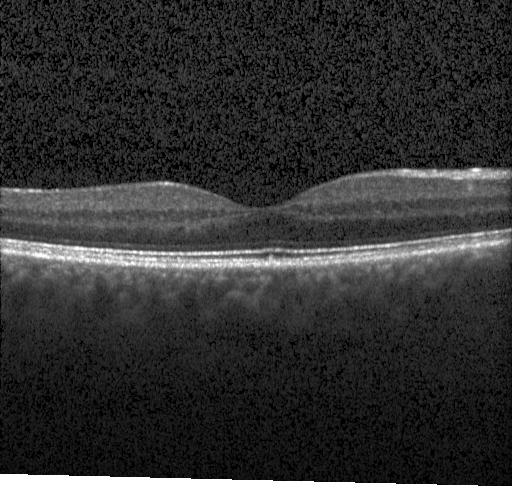 Retinal OCT B-scan — The scan shows neither choroidal neovascularization, diabetic macular edema, nor drusen.